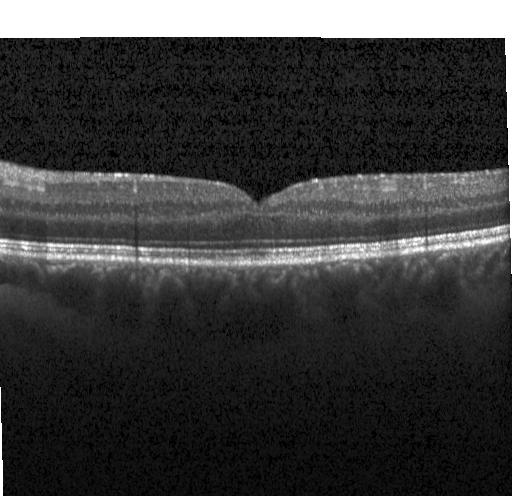

Spectral-domain OCT, OCT line scan, centered on the fovea, Heidelberg Spectralis OCT system. This B-scan demonstrates no choroidal neovascularization, no diabetic macular edema, and no drusen.